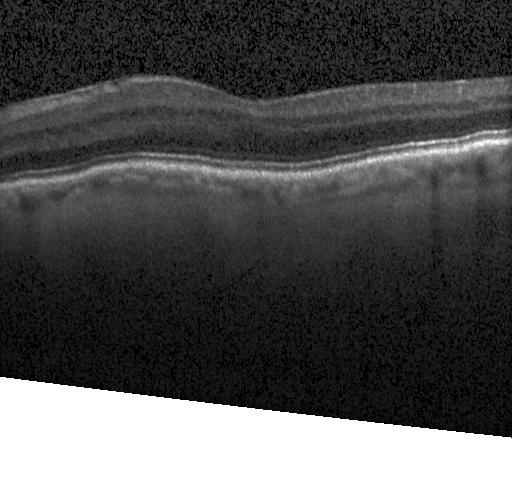
No evidence of CNV, DME, or drusen.